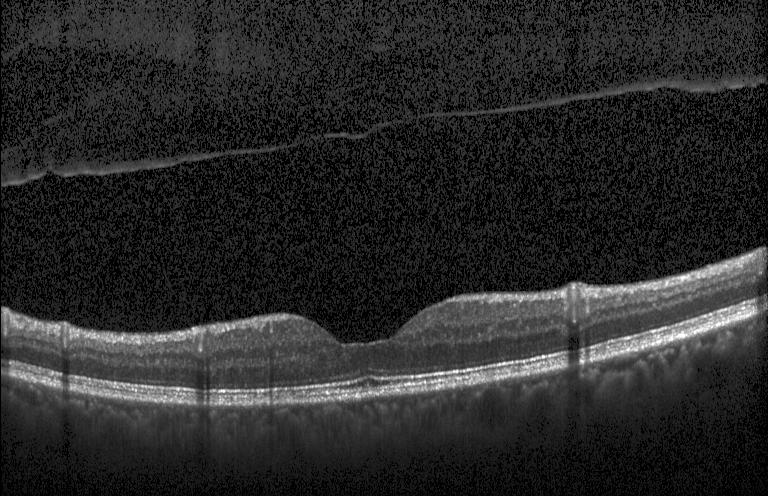
Heidelberg Spectralis OCT system, retinal OCT B-scan, spectral-domain OCT
Finding: no choroidal neovascularization, no diabetic macular edema, and no drusen.